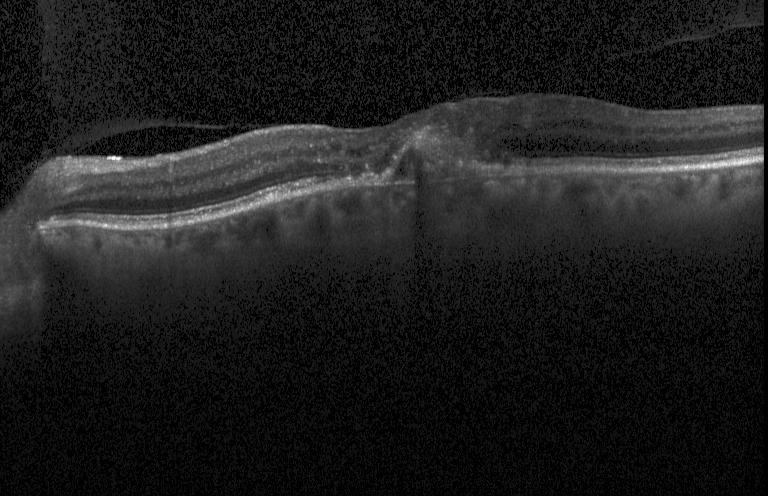 OCT B-scan showing a choroidal neovascular membrane.